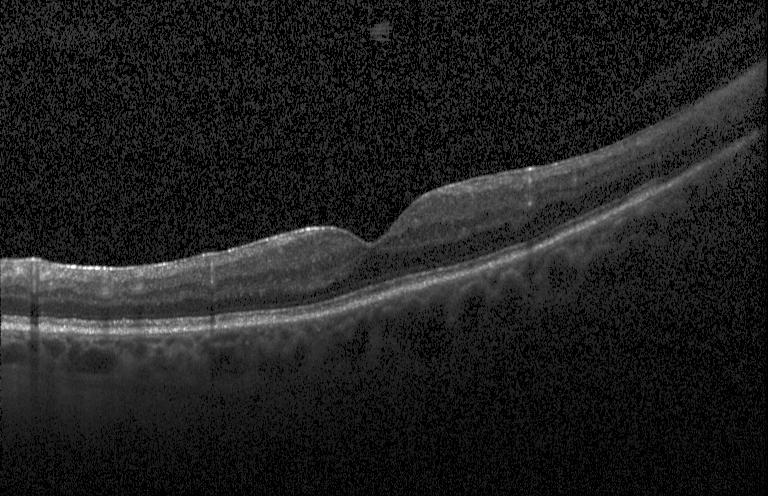 This B-scan demonstrates no evidence of choroidal neovascularization, diabetic macular edema, or drusen.